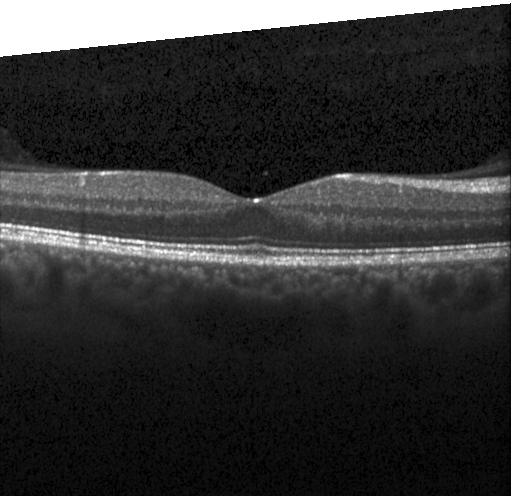 Spectral-domain optical coherence tomography, fovea-centered, retinal OCT cross-section — The scan shows no evidence of choroidal neovascularization, diabetic macular edema, or drusen.